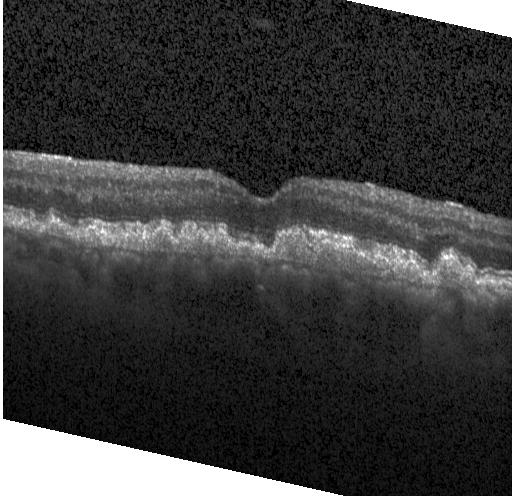

Spectral-domain optical coherence tomography. Macular scan. Acquired on a Heidelberg Spectralis. Optical coherence tomography B-scan. This B-scan demonstrates a choroidal neovascular membrane.